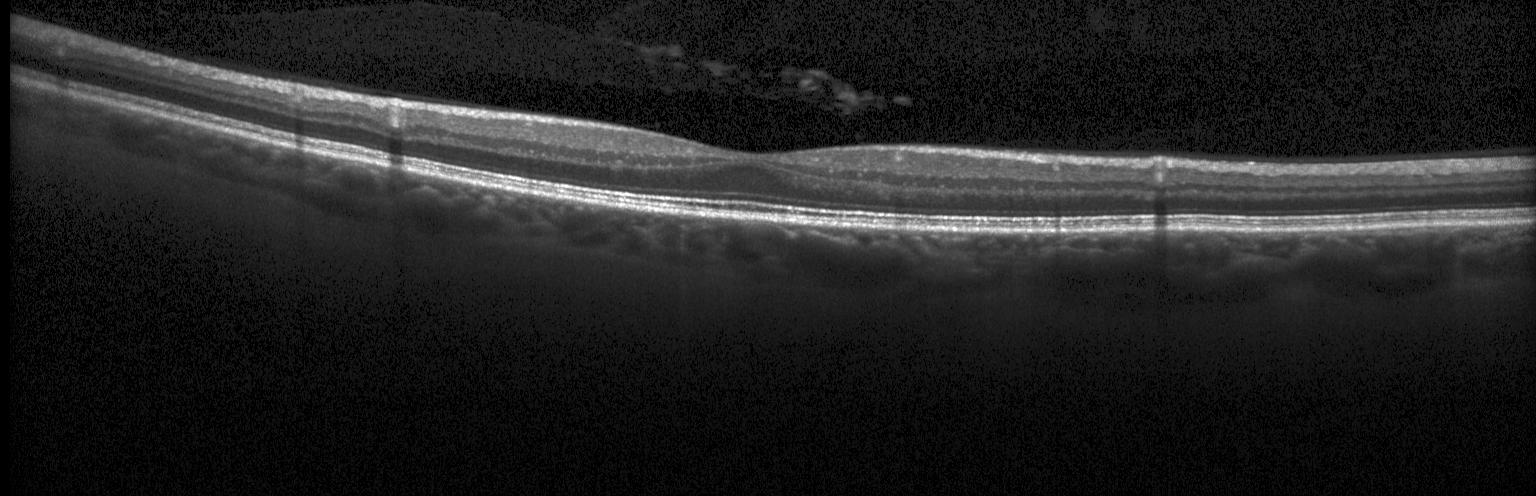

Macular OCT demonstrating no evidence of choroidal neovascularization, diabetic macular edema, or drusen.